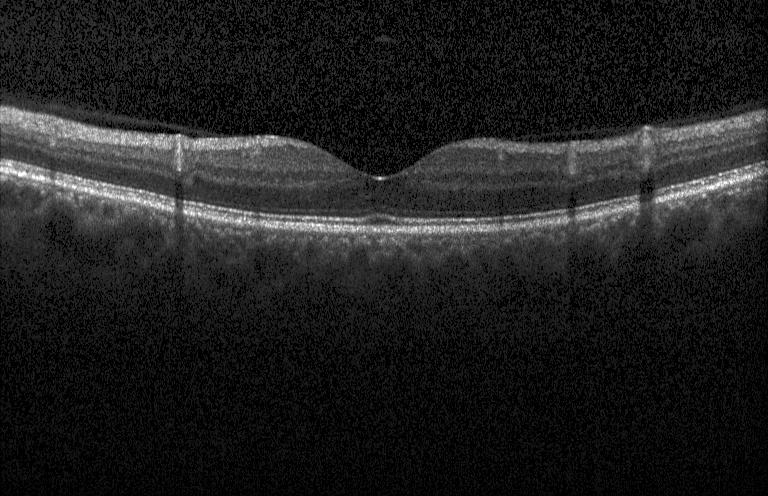
Dx: no CNV, no DME, and no drusen.